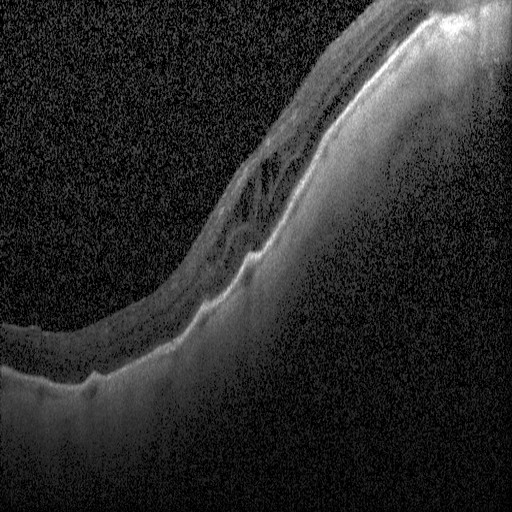

OCT B-scan showing diabetic macular edema (DME).